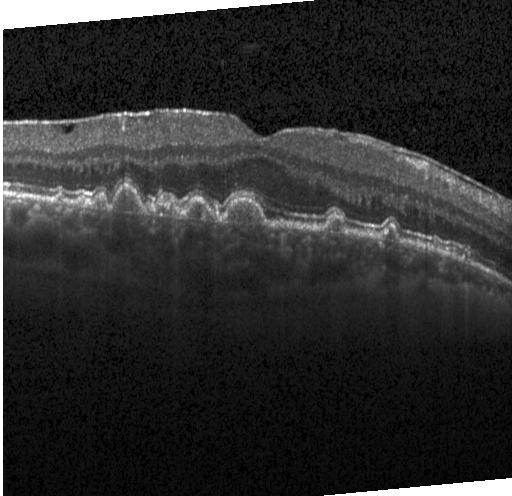

OCT line scan. Instrument: Heidelberg Spectralis. Fovea-centered.
Finding: drusen.